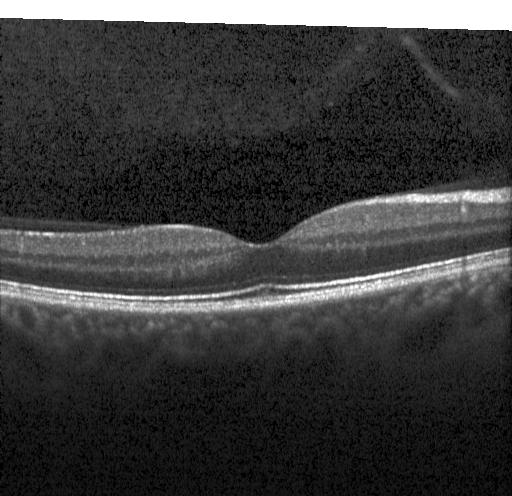
OCT B-scan showing neither choroidal neovascularization, diabetic macular edema, nor drusen.